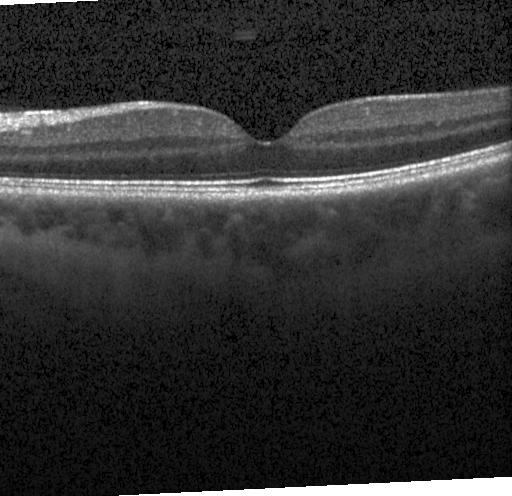

OCT B-scan
Diagnosis: no choroidal neovascularization, no diabetic macular edema, and no drusen.